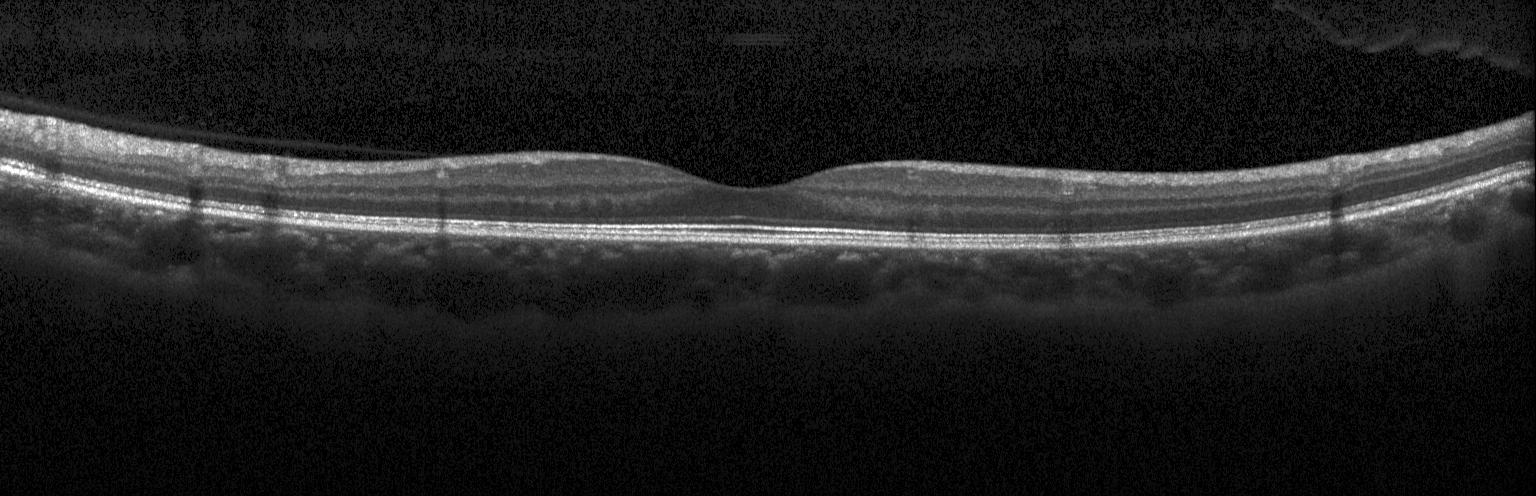

Spectral-domain OCT; retinal OCT B-scan; centered on the fovea
Diagnosis: neither choroidal neovascularization, diabetic macular edema, nor drusen.